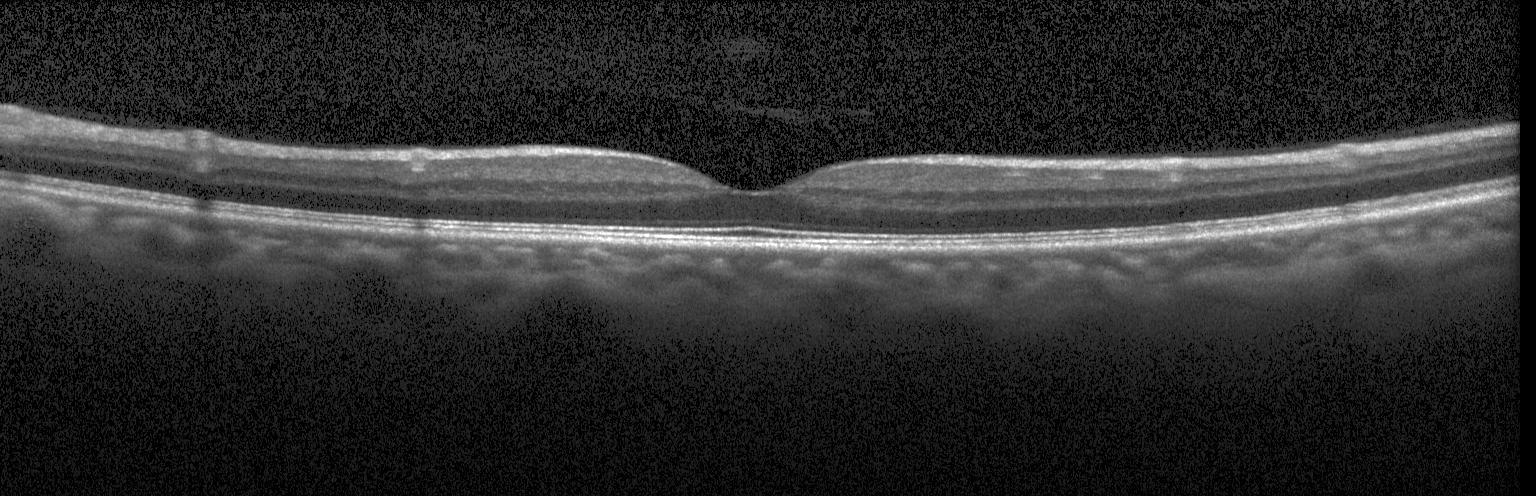
Macular scan · spectral-domain OCT · OCT line scan — Macular OCT: no evidence of choroidal neovascularization, diabetic macular edema, or drusen.